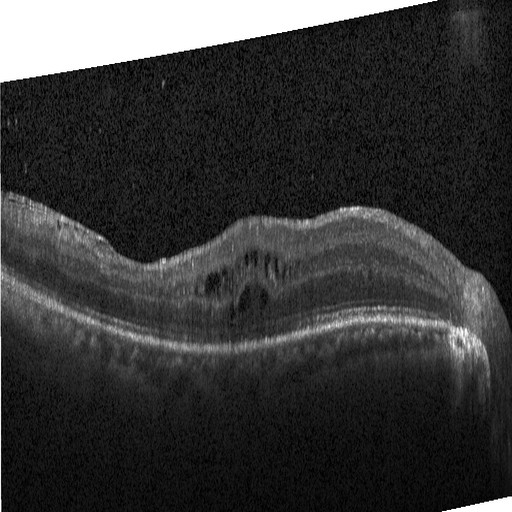

Macular scan; retinal OCT cross-section; instrument: Heidelberg Spectralis. Assessment: DME.